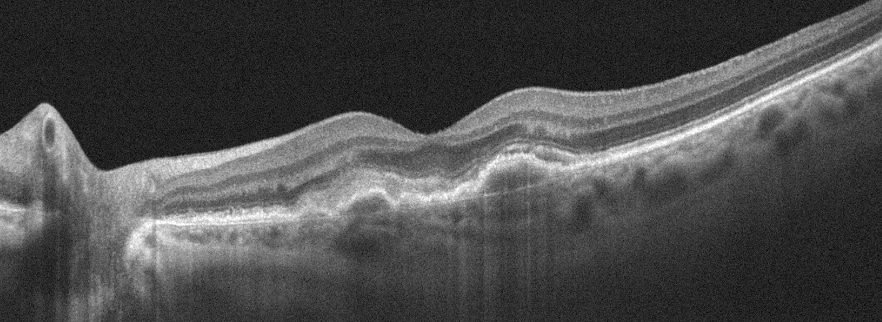 Retinal OCT cross-section · left eye — Age-related macular degeneration (AMD).